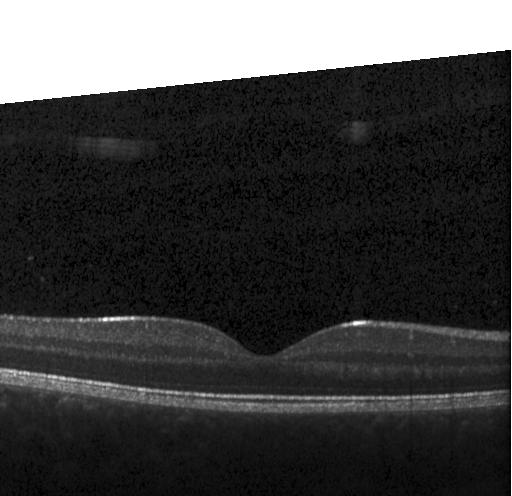 Optical coherence tomography B-scan · spectral-domain OCT · horizontal scan through the fovea — Macular OCT: no evidence of choroidal neovascularization, diabetic macular edema, or drusen.